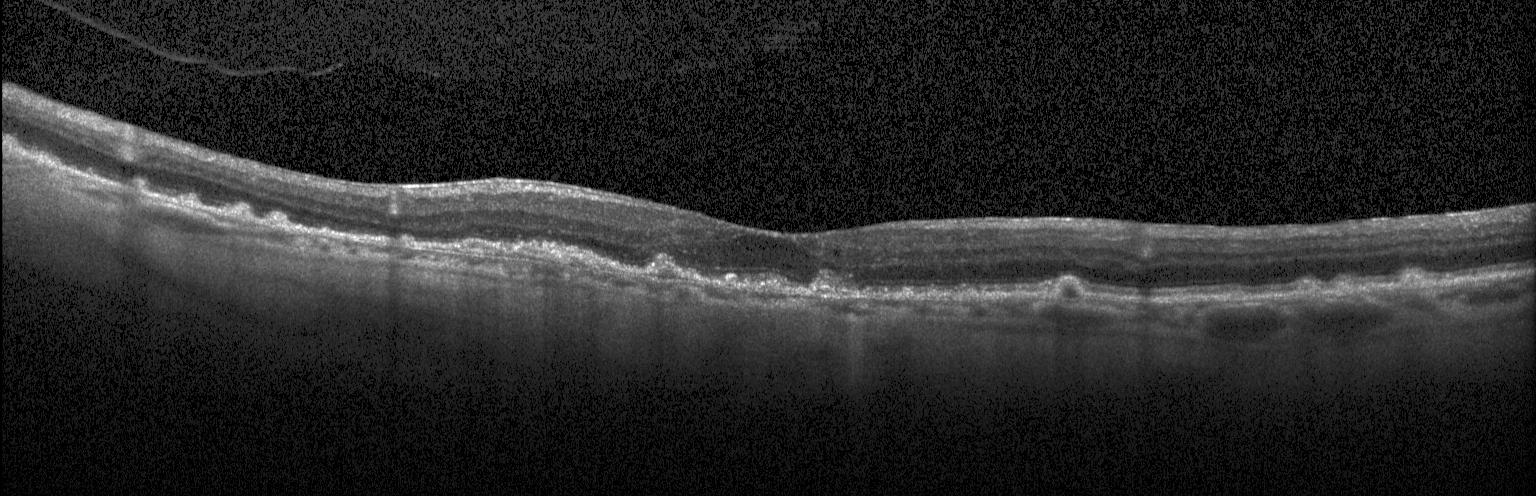 Retinal OCT cross-section showing choroidal neovascularization.